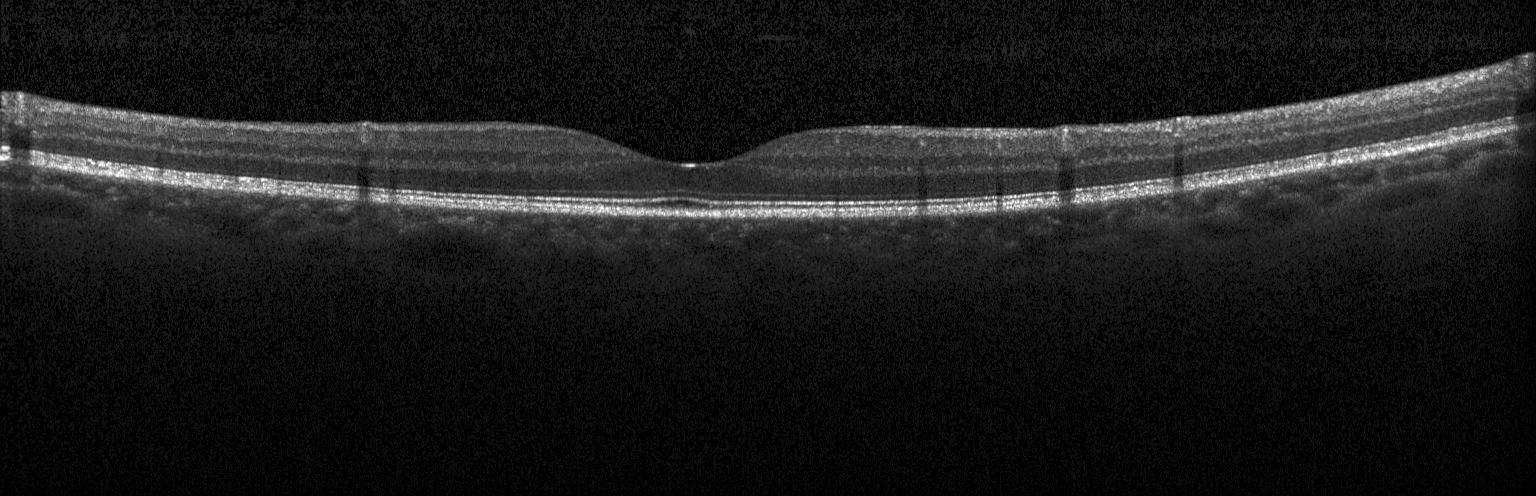
Assessment: no evidence of choroidal neovascularization, diabetic macular edema, or drusen.